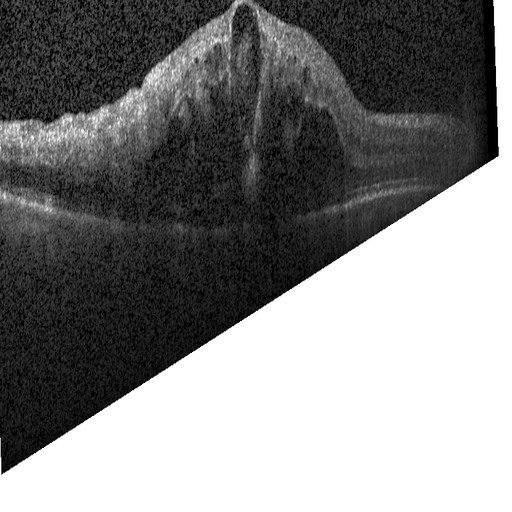 Optical coherence tomography scan. Spectral-domain OCT. Heidelberg Spectralis OCT system — Assessment: diabetic macular edema.